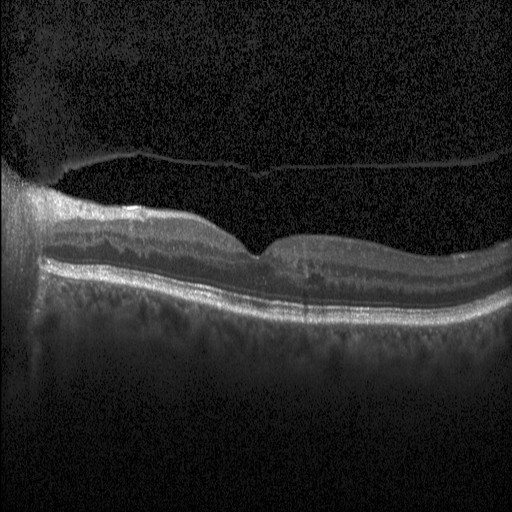 Optical coherence tomography scan · Heidelberg Spectralis OCT system · through the macula. Dx: diabetic macular edema.